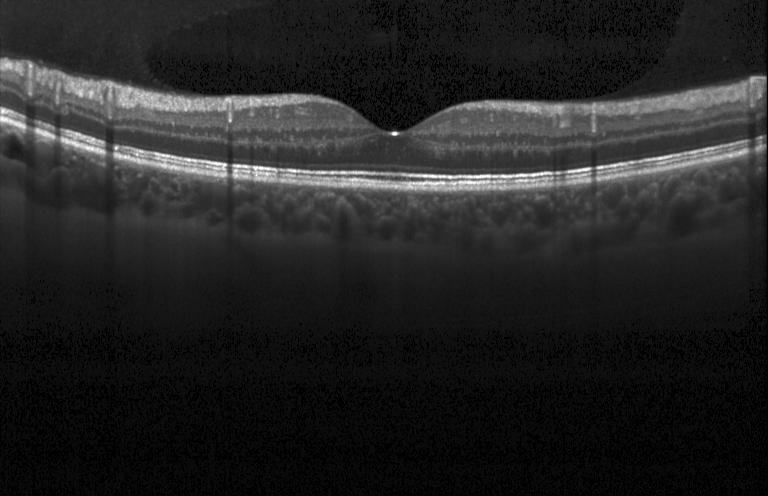

Impression: neither CNV, DME, nor drusen.